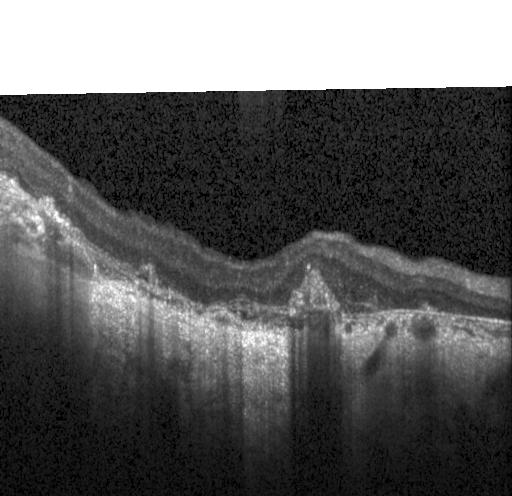 SD-OCT; retinal OCT cross-section — Finding: a choroidal neovascular membrane.